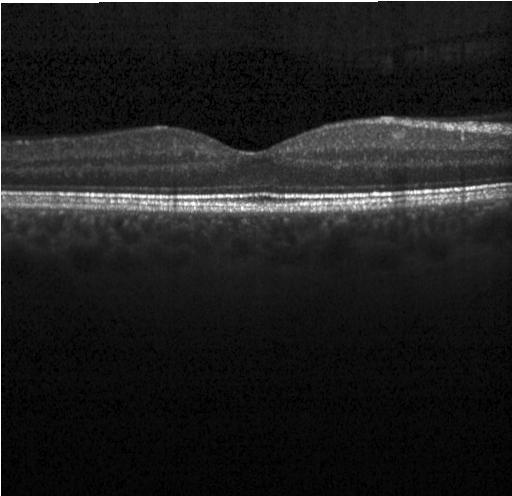

Retinal OCT B-scan. Impression: no CNV, no DME, and no drusen.